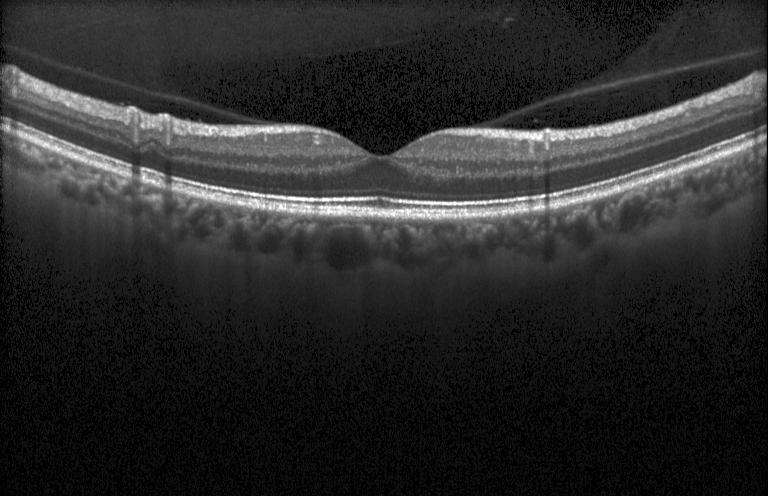

OCT line scan; spectral-domain OCT — Dx: neither CNV, DME, nor drusen.